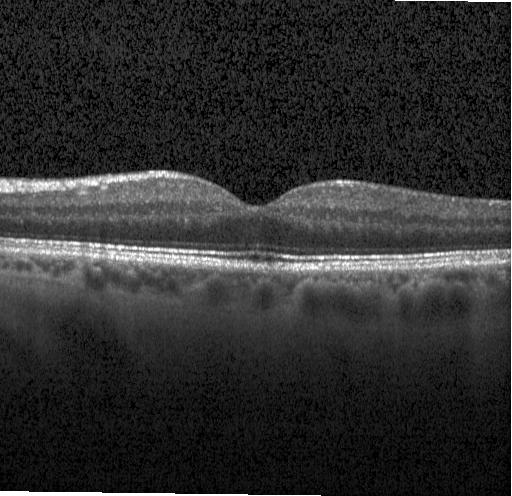 Spectral-domain optical coherence tomography; OCT line scan
OCT finding: no evidence of CNV, DME, or drusen.